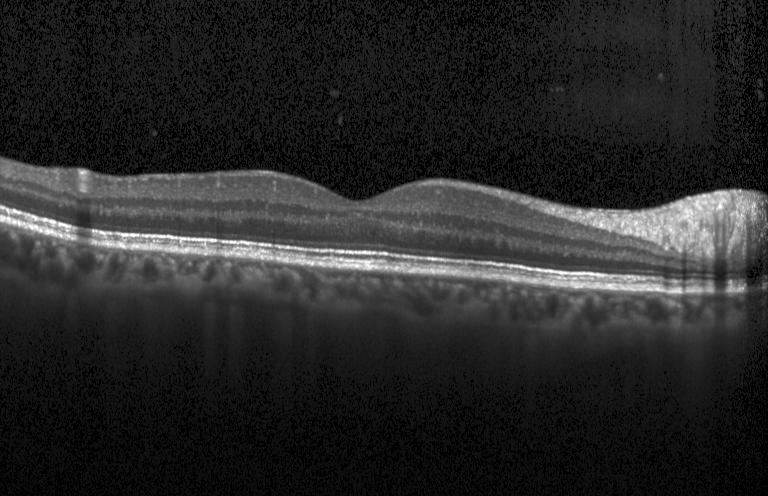
Macular OCT: no choroidal neovascularization, no diabetic macular edema, and no drusen.